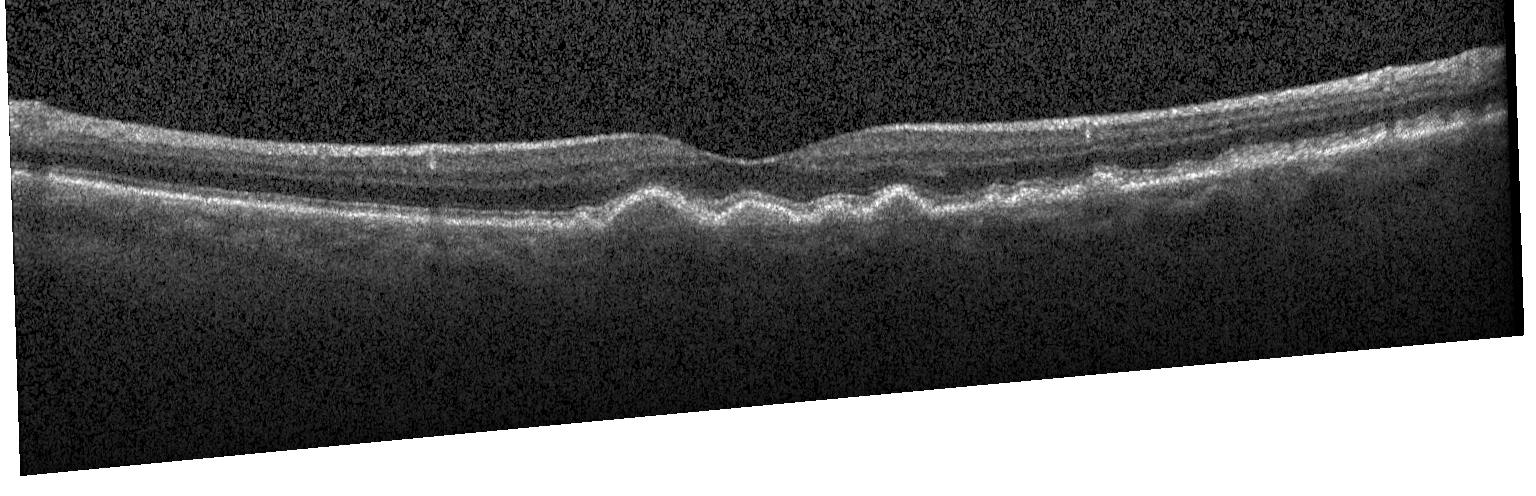
Macular scan · retinal OCT cross-section.
Diagnosis: multiple drusen.